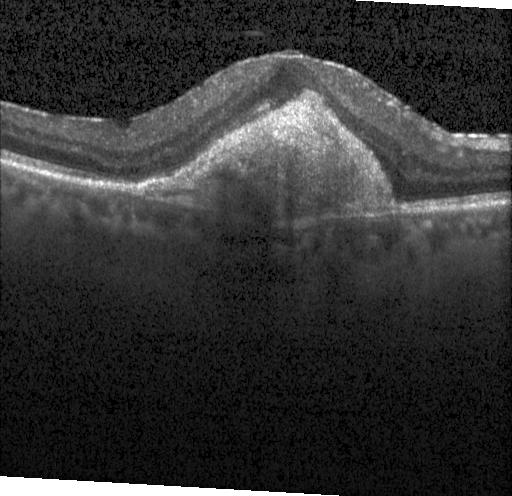 Instrument: Heidelberg Spectralis. OCT B-scan. Horizontal scan through the fovea
Finding: a choroidal neovascular membrane.